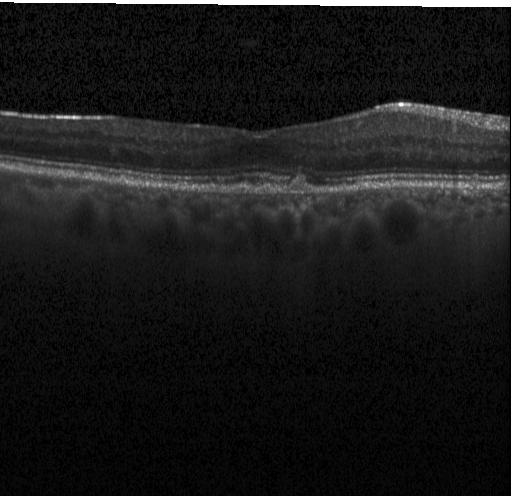 Retinal OCT B-scan · SD-OCT · macular scan
Dx: sub-RPE drusenoid deposits.